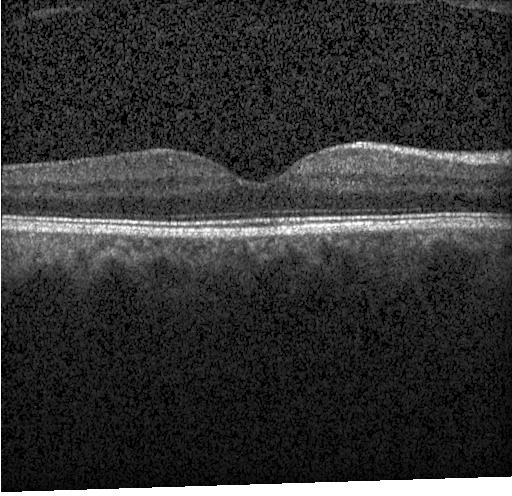 Horizontal scan through the fovea, optical coherence tomography B-scan, spectral-domain OCT
Diagnosis: no choroidal neovascularization, no diabetic macular edema, and no drusen.